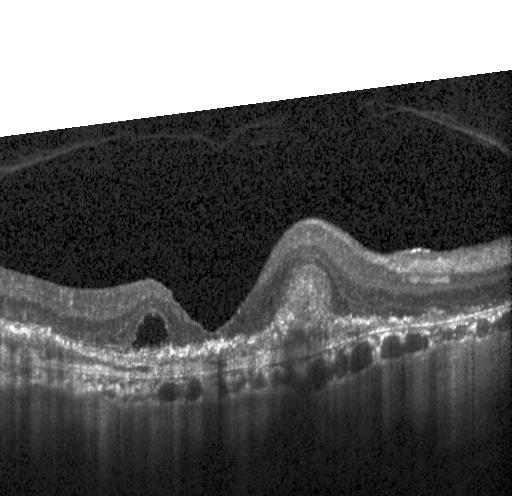
CNV.